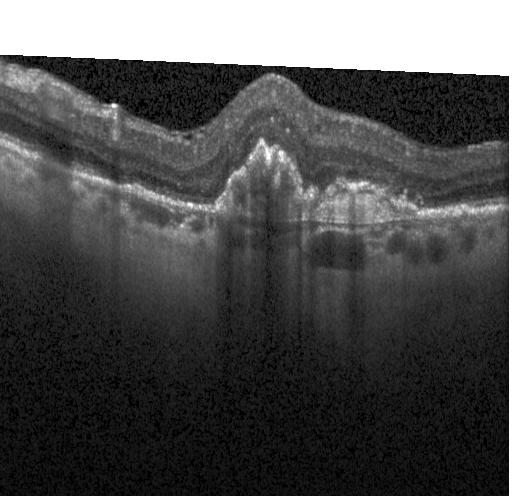 Horizontal scan through the fovea · retinal OCT B-scan · spectral-domain optical coherence tomography · Heidelberg Spectralis OCT system.
The scan shows a choroidal neovascular membrane.